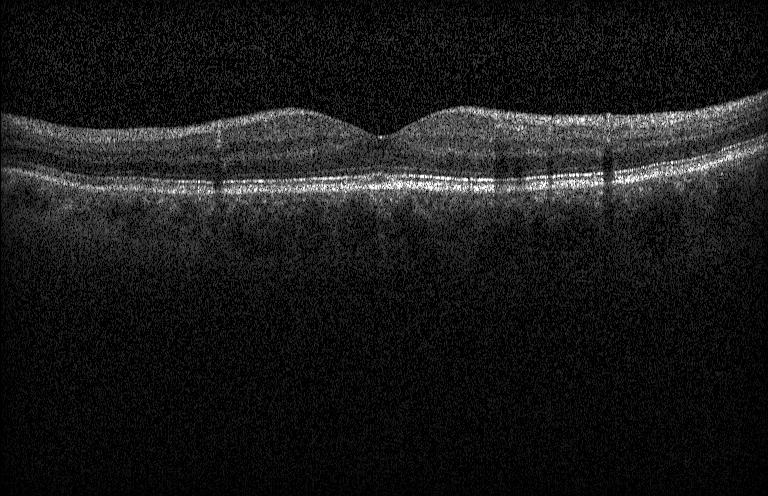

OCT line scan — Dx: neither choroidal neovascularization, diabetic macular edema, nor drusen.